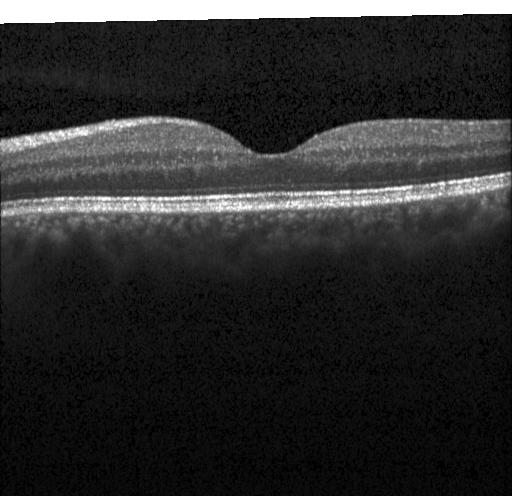

Neither choroidal neovascularization, diabetic macular edema, nor drusen.